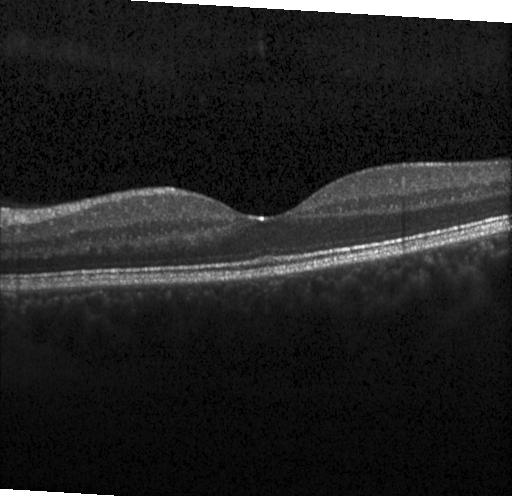
Heidelberg Spectralis; optical coherence tomography B-scan; spectral-domain optical coherence tomography; centered on the fovea. Dx: no CNV, no DME, and no drusen.